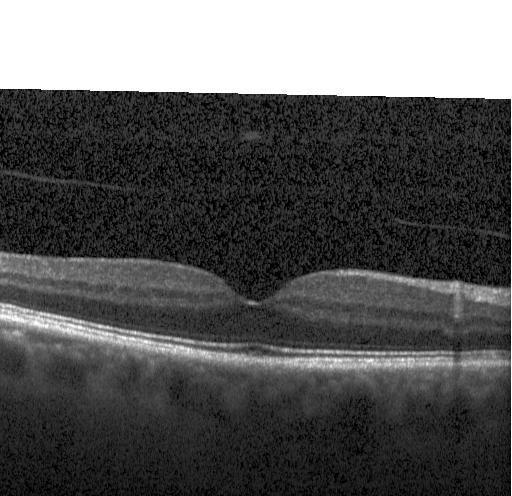
Spectral-domain OCT. Centered on the fovea. Heidelberg Spectralis OCT system. OCT line scan. Impression: no choroidal neovascularization, no diabetic macular edema, and no drusen.